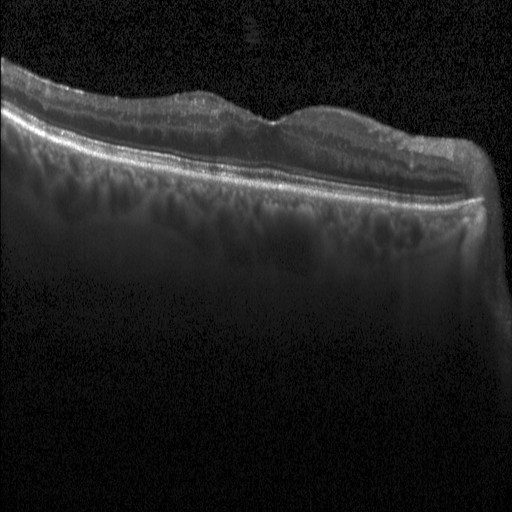
OCT B-scan showing diabetic macular edema (DME).